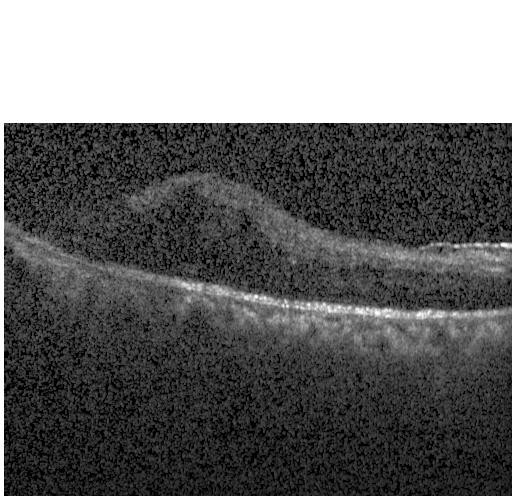

Diagnosis: DME.